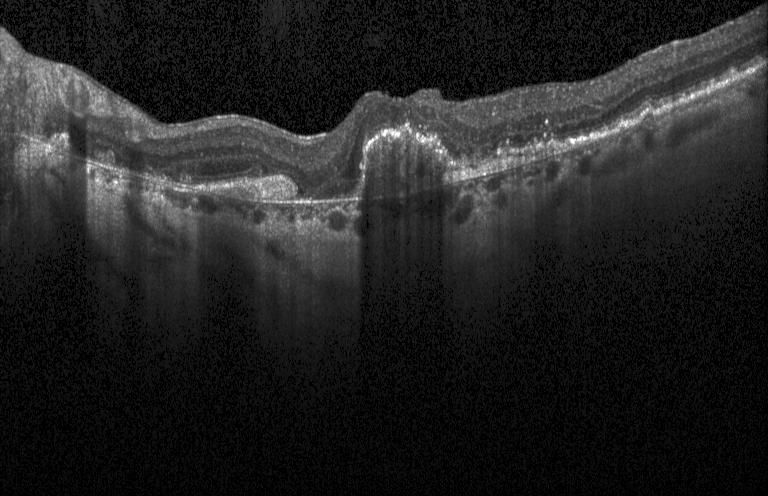

Retinal OCT cross-section — Assessment: CNV.